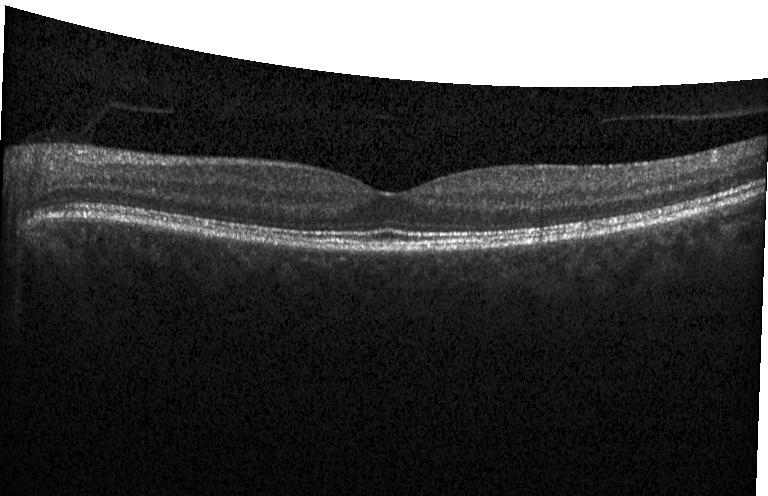

The scan shows no evidence of choroidal neovascularization, diabetic macular edema, or drusen.